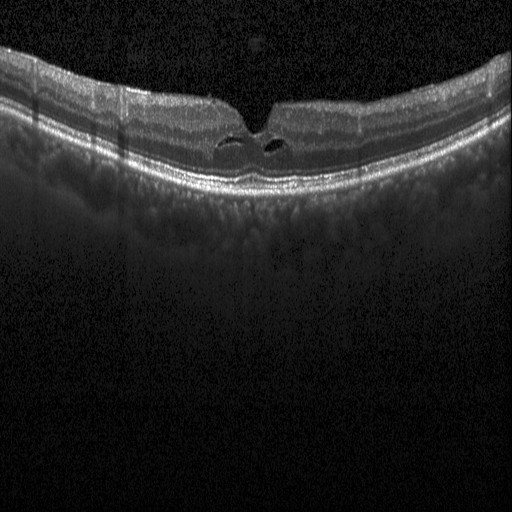
This B-scan demonstrates diabetic macular edema.